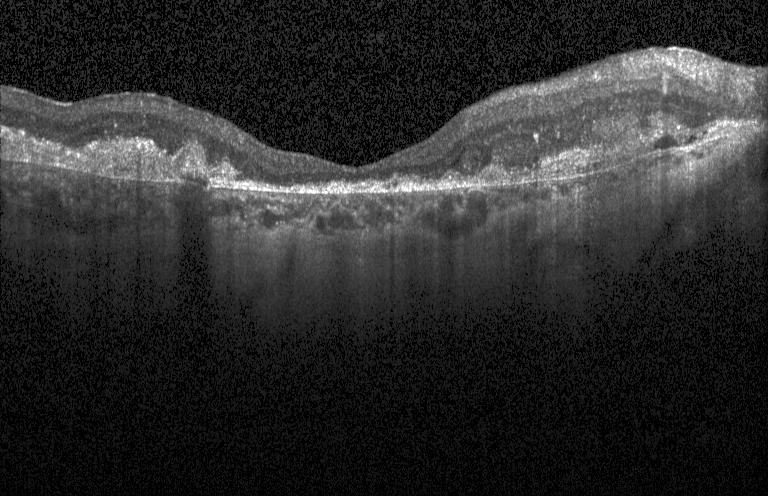 Optical coherence tomography scan. Spectral-domain optical coherence tomography.
Diagnosis: CNV.